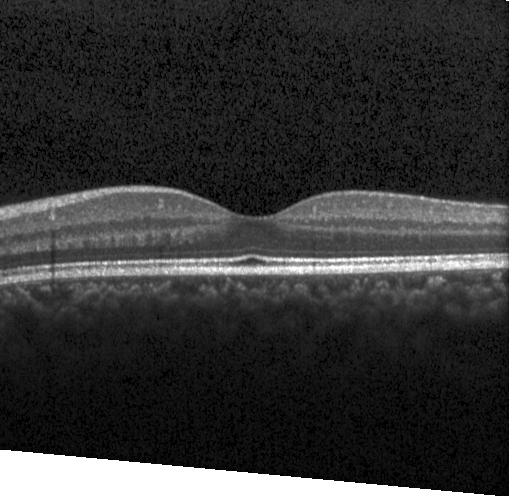
Acquired on a Heidelberg Spectralis, optical coherence tomography scan
Finding: no evidence of choroidal neovascularization, diabetic macular edema, or drusen.